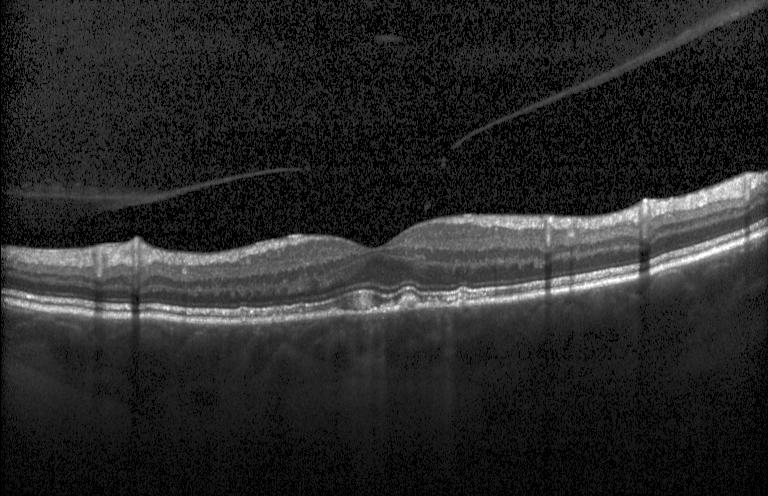 Retinal OCT cross-section
Diagnosis: drusen.